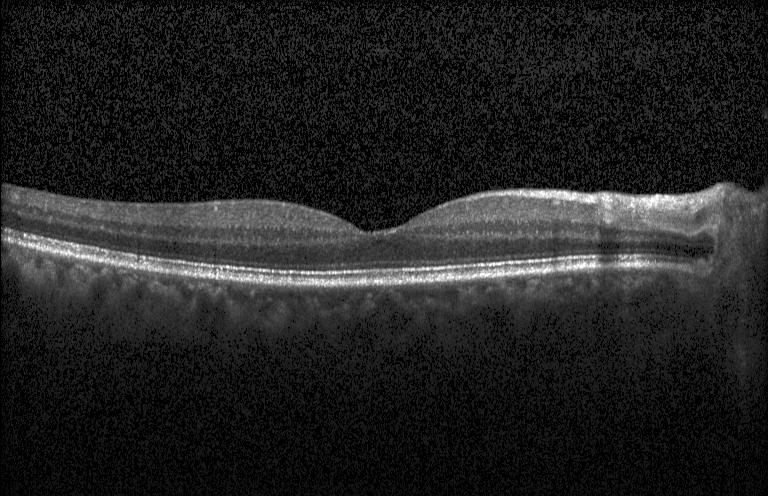

Finding: neither choroidal neovascularization, diabetic macular edema, nor drusen.